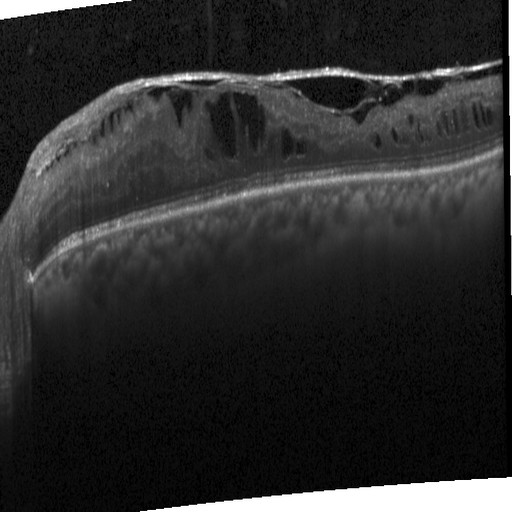
OCT B-scan showing diabetic macular edema.